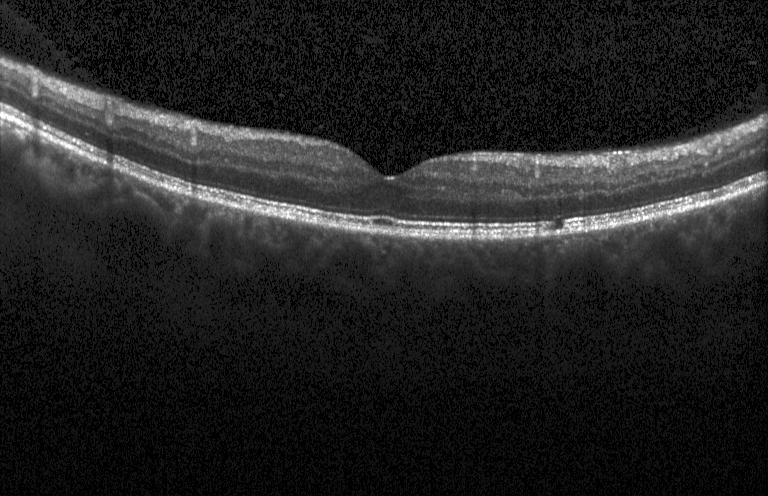

Optical coherence tomography scan. Diagnosis: no choroidal neovascularization, diabetic macular edema, or drusen.